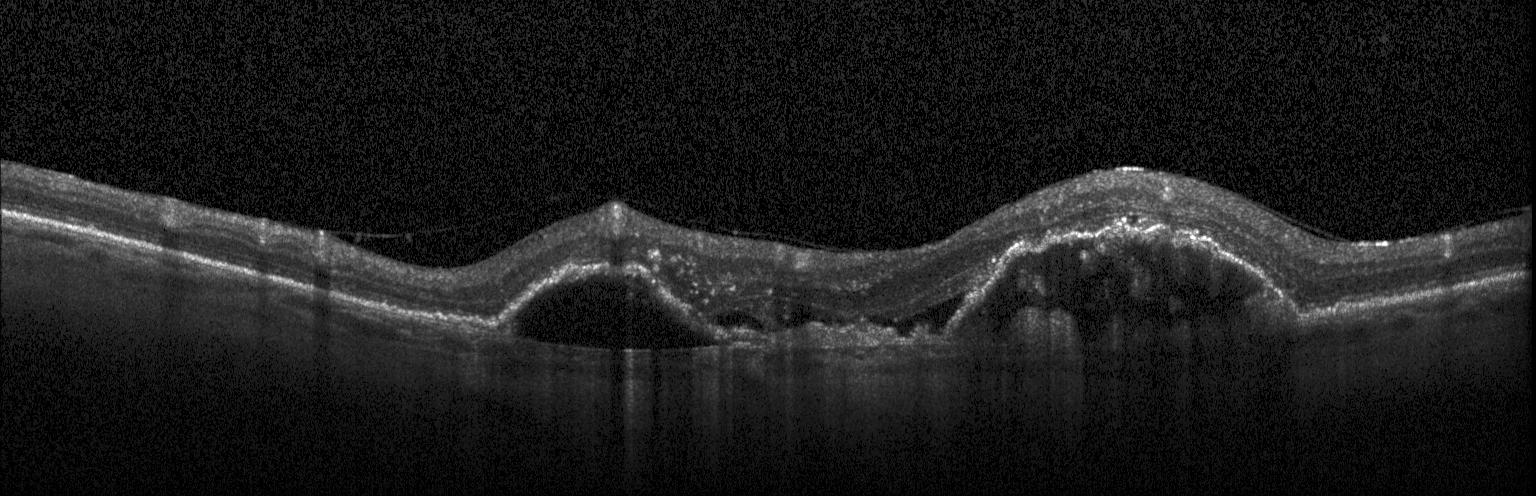

Heidelberg Spectralis · optical coherence tomography scan — Dx: choroidal neovascularization.